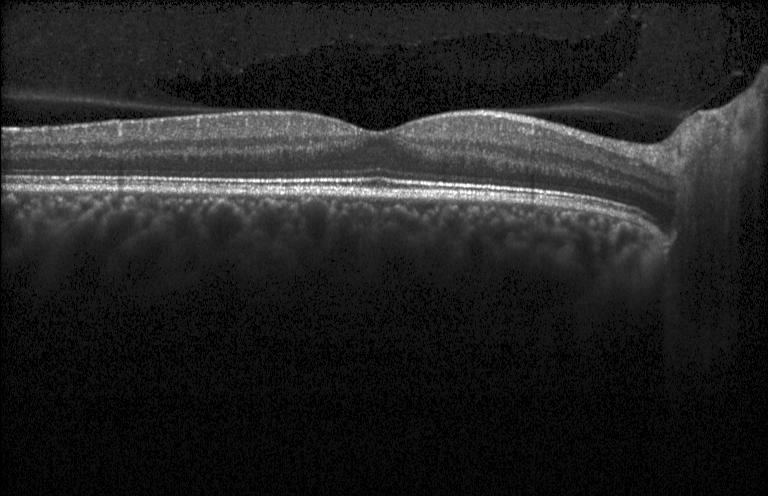

Retinal OCT cross-section showing no choroidal neovascularization, diabetic macular edema, or drusen.